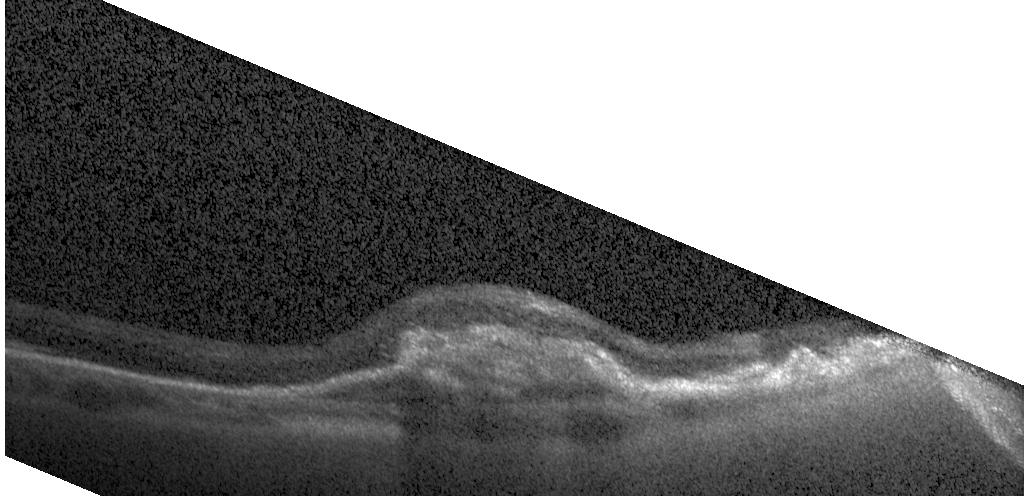
OCT B-scan showing a choroidal neovascular membrane.